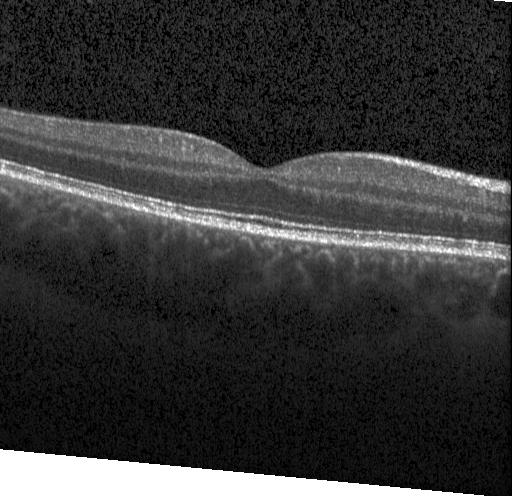
OCT B-scan · centered on the fovea · spectral-domain optical coherence tomography · instrument: Heidelberg Spectralis — Finding: no evidence of CNV, DME, or drusen.